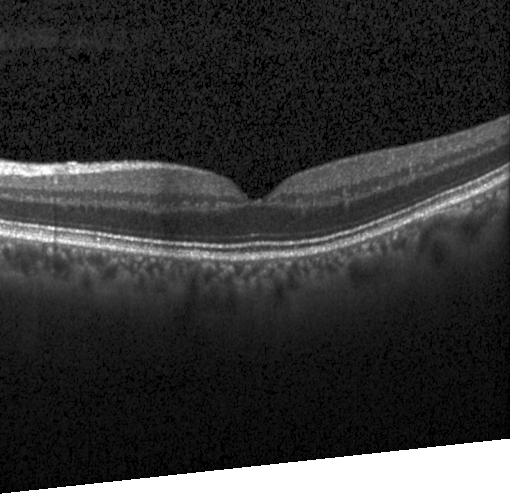

Centered on the fovea, instrument: Heidelberg Spectralis, OCT line scan — Impression: no choroidal neovascularization, no diabetic macular edema, and no drusen.